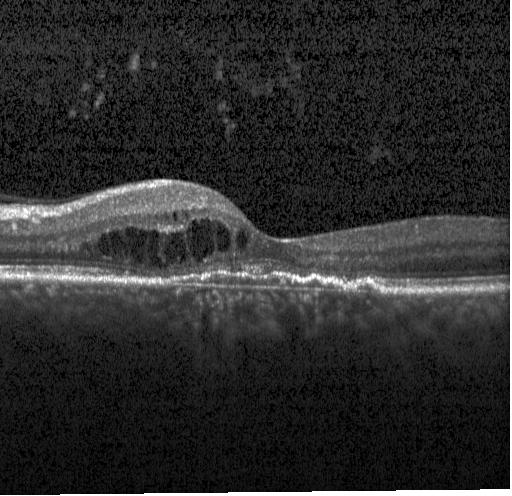
Optical coherence tomography scan. SD-OCT. Acquired on a Heidelberg Spectralis — Choroidal neovascularization.